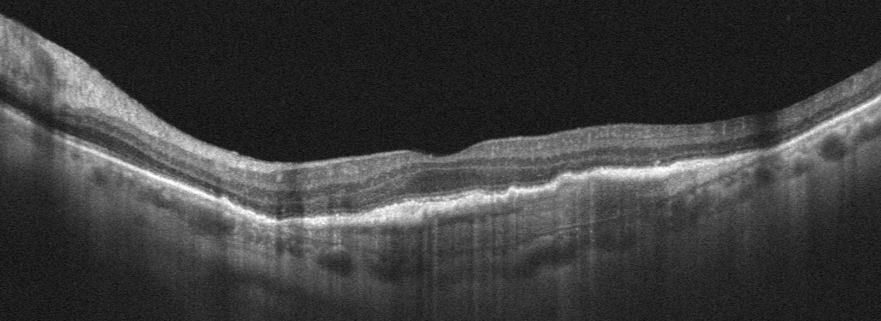
Acquired on an Optovue Avanti RTVue XR. Through the macula. OCT line scan
Age-related macular degeneration.